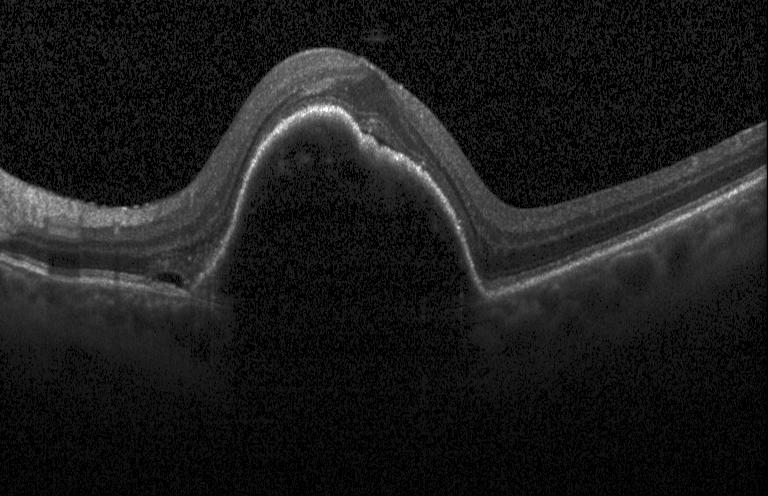

Through the macula. Heidelberg Spectralis OCT system. Retinal OCT cross-section
Dx: a choroidal neovascular membrane.